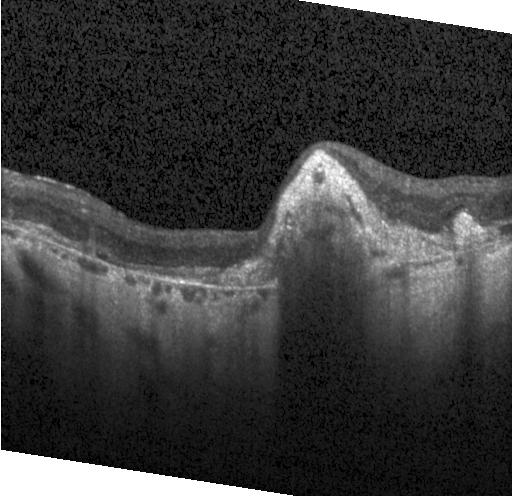
Fovea-centered, optical coherence tomography B-scan, spectral-domain optical coherence tomography — Assessment: choroidal neovascularization.